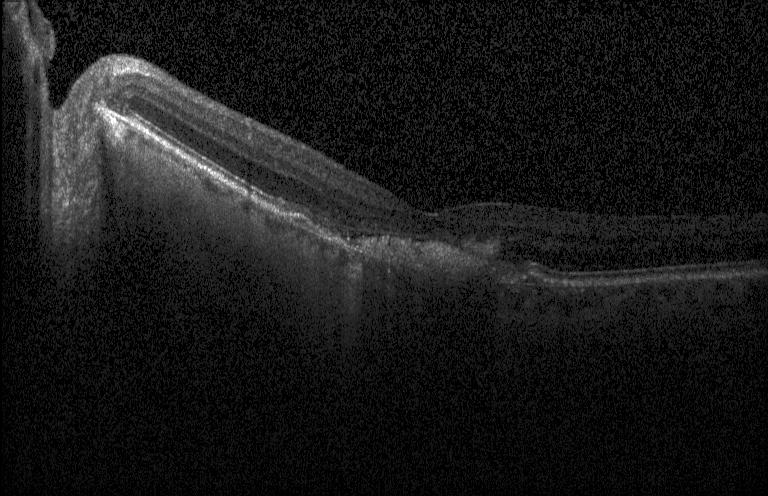
Through the macula · retinal OCT B-scan. Diagnosis: choroidal neovascularization.